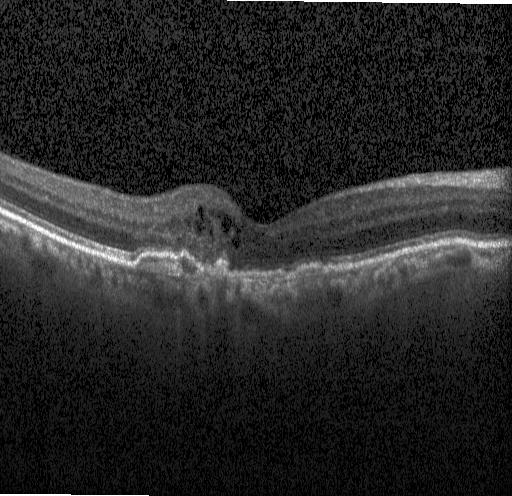
Spectral-domain optical coherence tomography · OCT line scan
The scan shows a choroidal neovascular membrane.